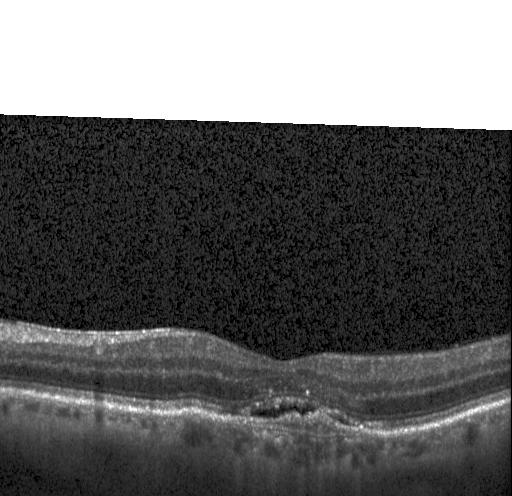 Optical coherence tomography scan. Impression: a choroidal neovascular membrane.